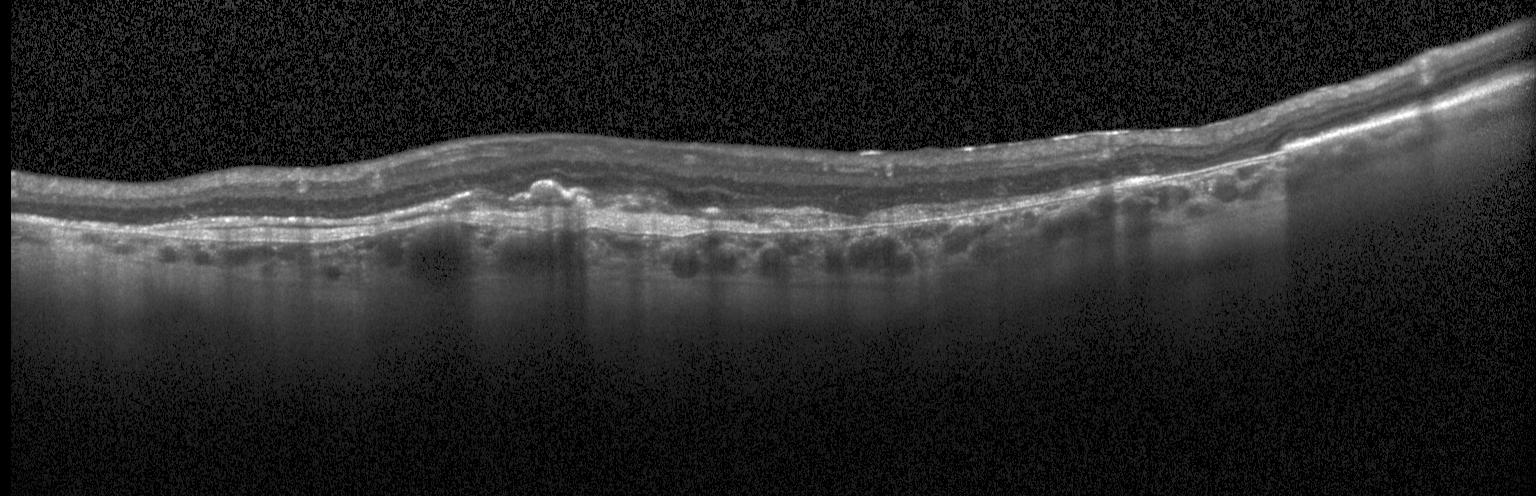
Finding: choroidal neovascularization.